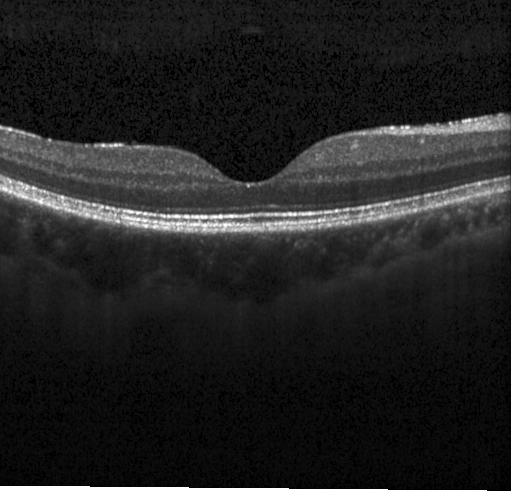

Optical coherence tomography B-scan · through the macula. Assessment: no choroidal neovascularization, diabetic macular edema, or drusen.